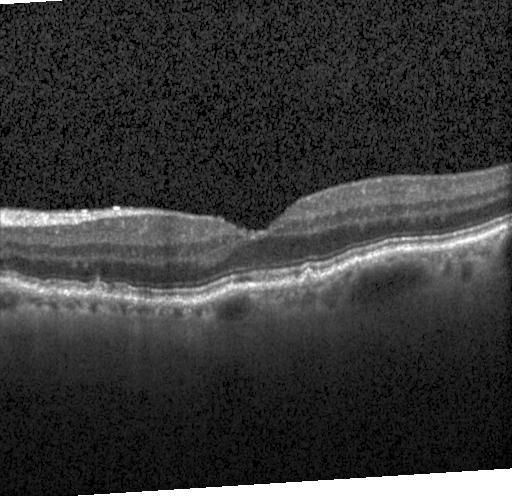 Retinal OCT B-scan. Macular scan. Spectral-domain optical coherence tomography.
Diagnosis: multiple drusen.